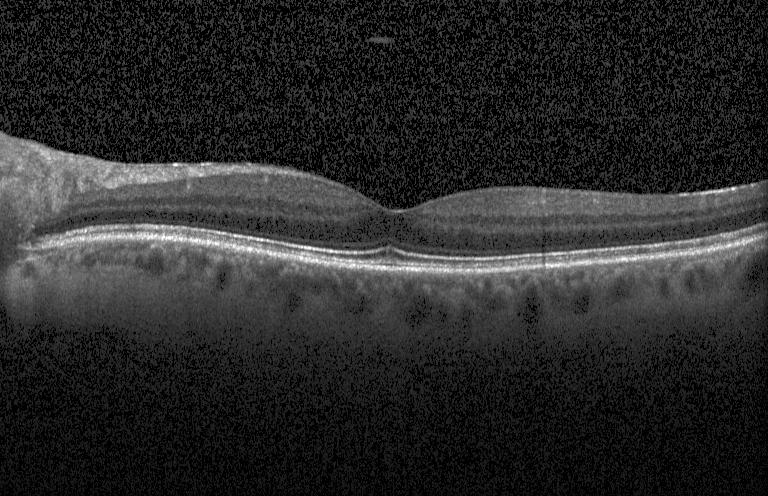
Horizontal scan through the fovea. Instrument: Heidelberg Spectralis. Retinal OCT cross-section.
OCT finding: neither CNV, DME, nor drusen.